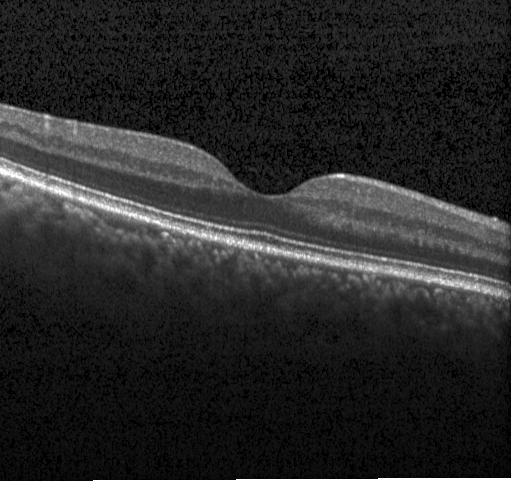
Optical coherence tomography scan
Diagnosis: neither choroidal neovascularization, diabetic macular edema, nor drusen.